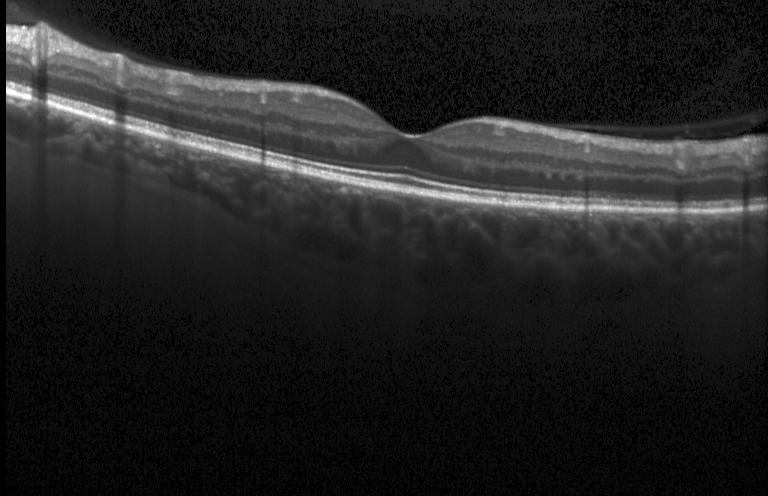
Macular OCT demonstrating no choroidal neovascularization, no diabetic macular edema, and no drusen.